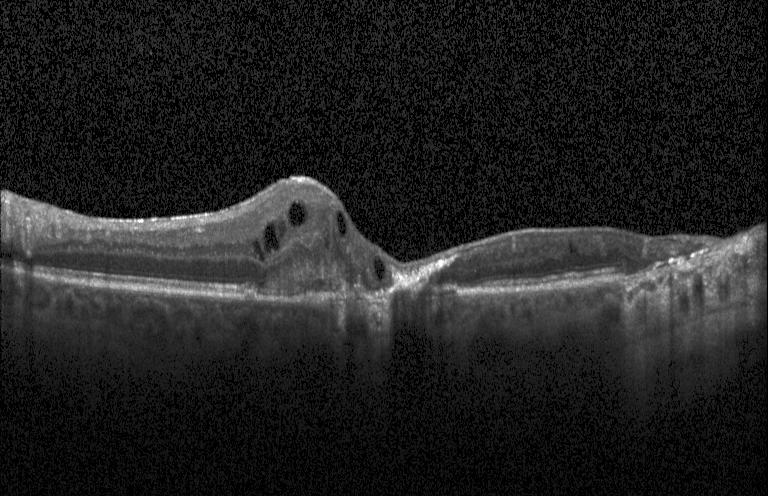 Spectral-domain optical coherence tomography. Retinal OCT cross-section. Through the macula
Finding: choroidal neovascularization (CNV).